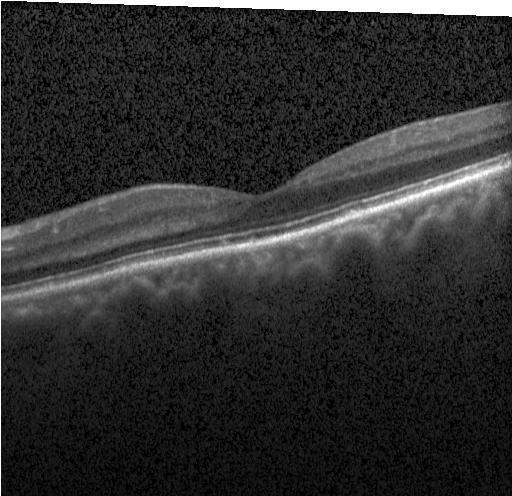

Dx: no choroidal neovascularization, diabetic macular edema, or drusen.